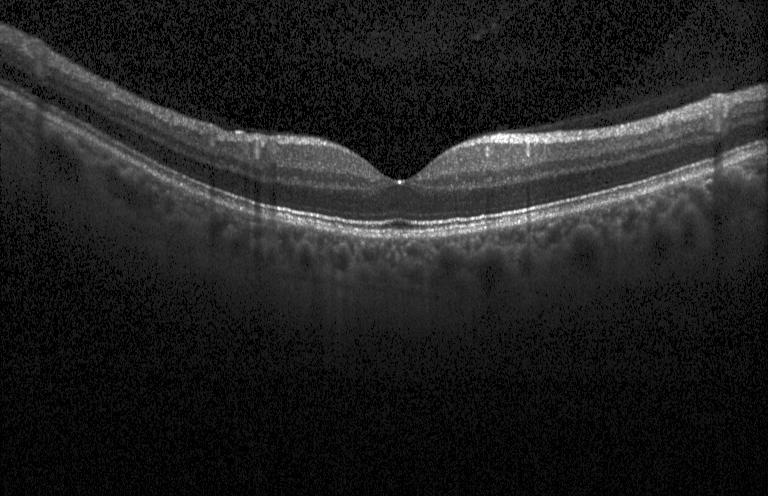

Neither choroidal neovascularization, diabetic macular edema, nor drusen.